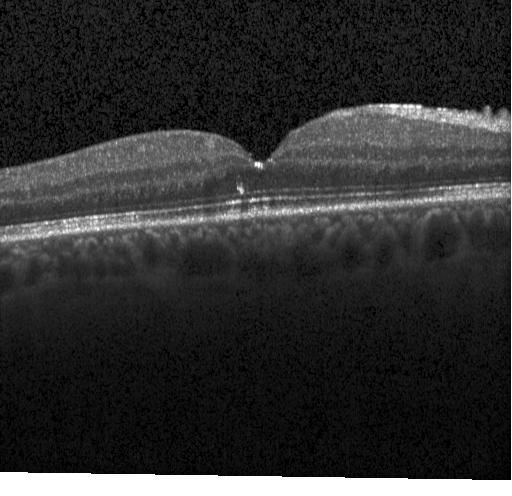

Heidelberg Spectralis · fovea-centered · retinal OCT cross-section. Assessment: no CNV, no DME, and no drusen.